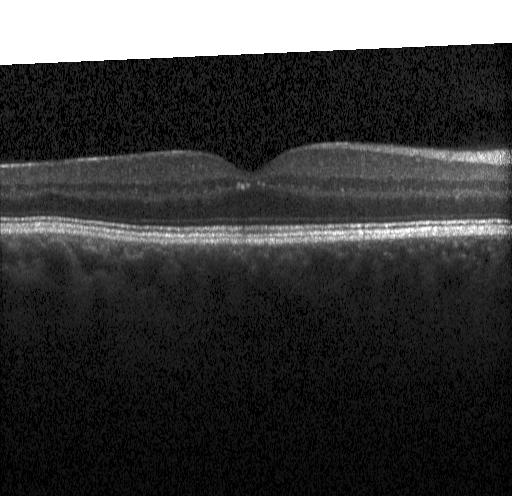

Diagnosis: neither choroidal neovascularization, diabetic macular edema, nor drusen.